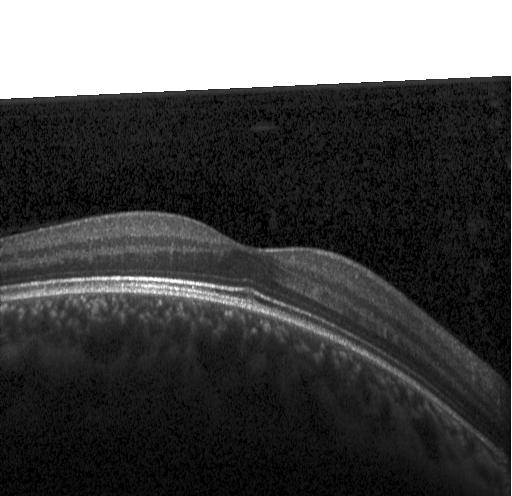
Impression: no evidence of choroidal neovascularization, diabetic macular edema, or drusen.